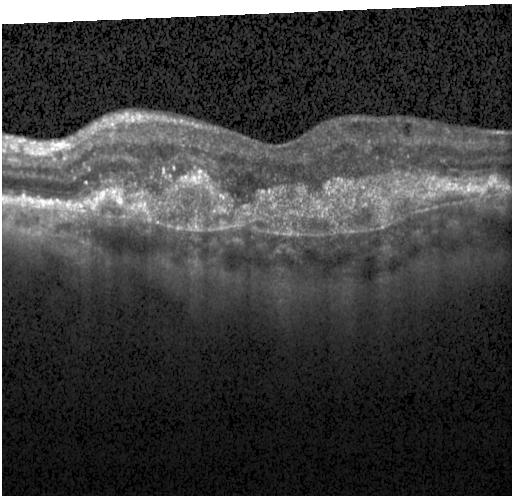 Spectral-domain optical coherence tomography, OCT B-scan, Heidelberg Spectralis — The scan shows CNV.